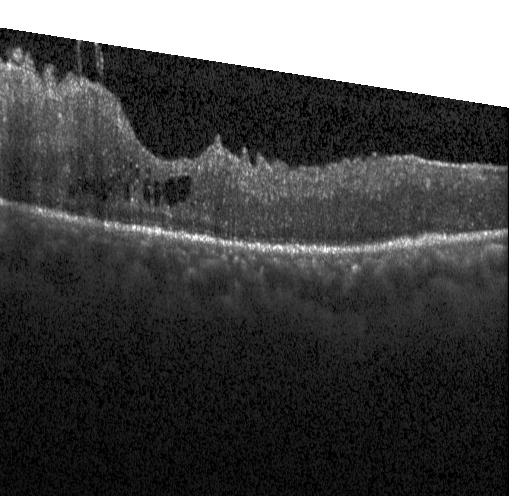
OCT B-scan.
DME.